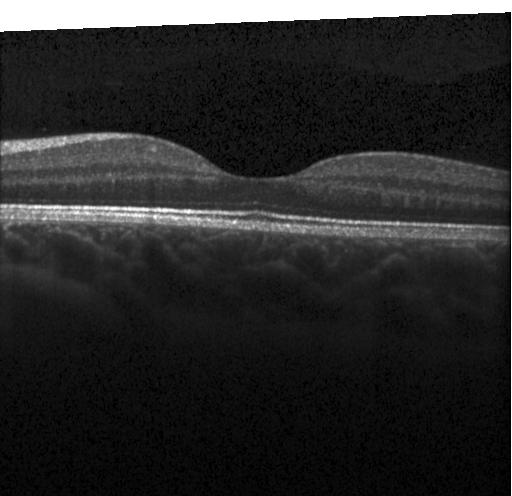

No choroidal neovascularization, no diabetic macular edema, and no drusen.